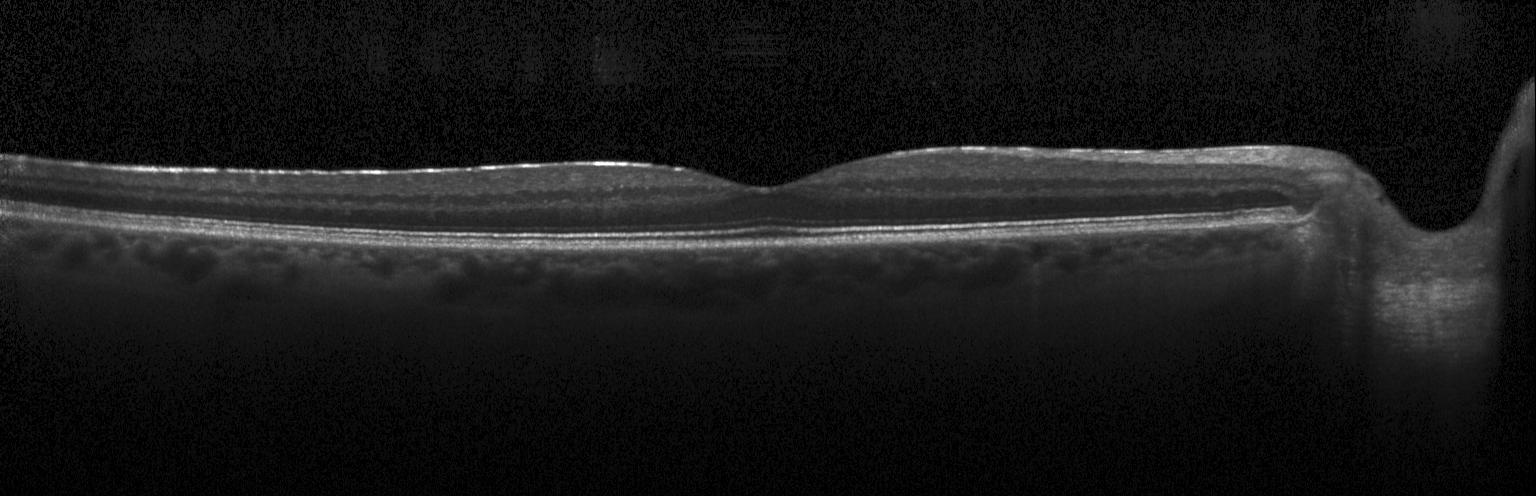 OCT line scan. Acquired on a Heidelberg Spectralis — OCT finding: no CNV, no DME, and no drusen.